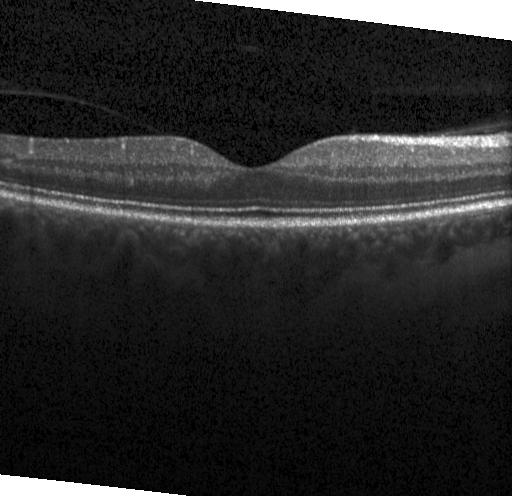
Spectral-domain optical coherence tomography; through the macula; instrument: Heidelberg Spectralis; retinal OCT cross-section.
Finding: no choroidal neovascularization, no diabetic macular edema, and no drusen.